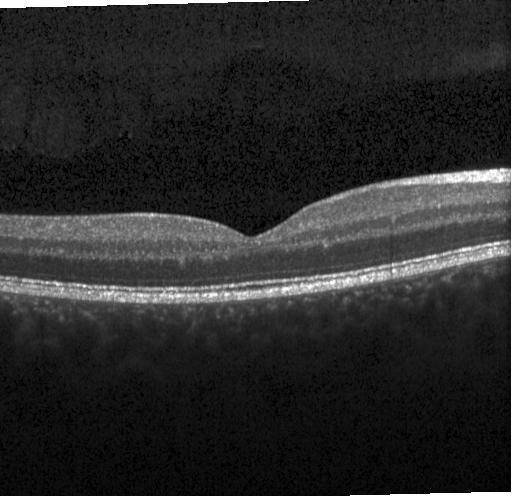 OCT line scan, Heidelberg Spectralis OCT system, horizontal scan through the fovea. OCT finding: no choroidal neovascularization, diabetic macular edema, or drusen.